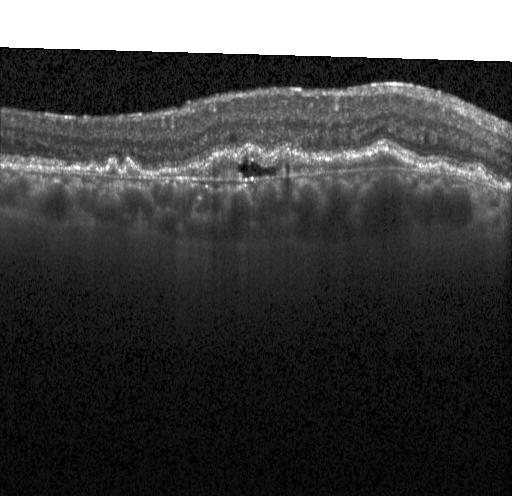
Assessment: a choroidal neovascular membrane.